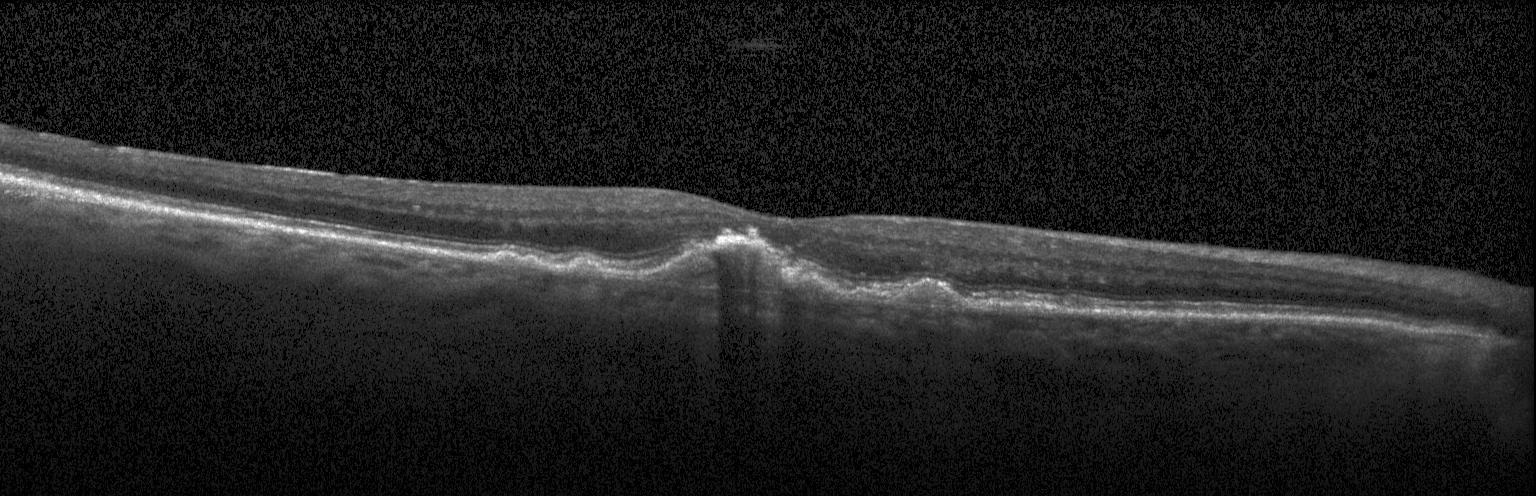
OCT scan showing a choroidal neovascular membrane.